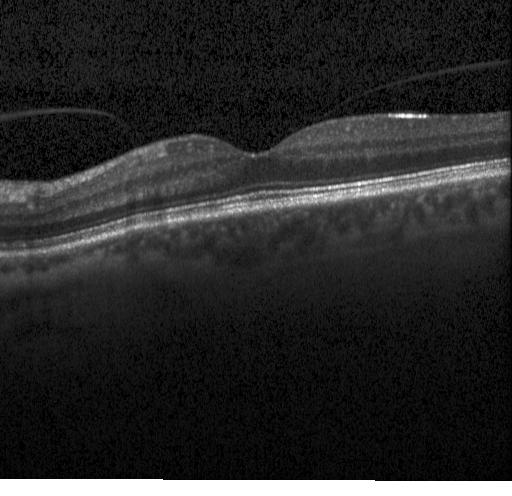 Dx: neither choroidal neovascularization, diabetic macular edema, nor drusen.